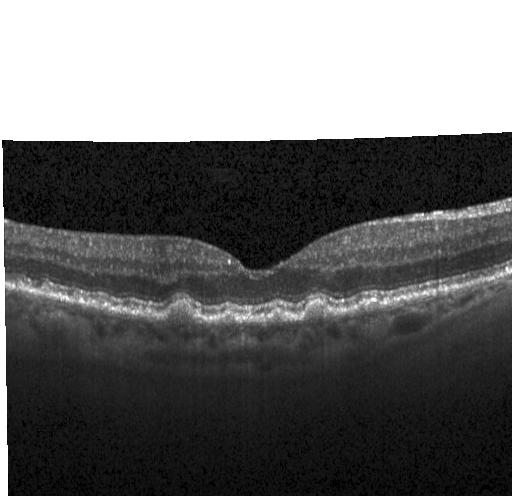

Optical coherence tomography scan. Horizontal scan through the fovea. Spectral-domain OCT — Sub-RPE drusenoid deposits.